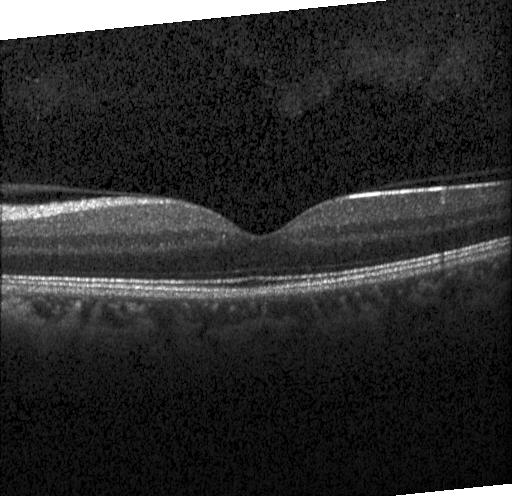 OCT B-scan, instrument: Heidelberg Spectralis, horizontal scan through the fovea
Diagnosis: neither CNV, DME, nor drusen.